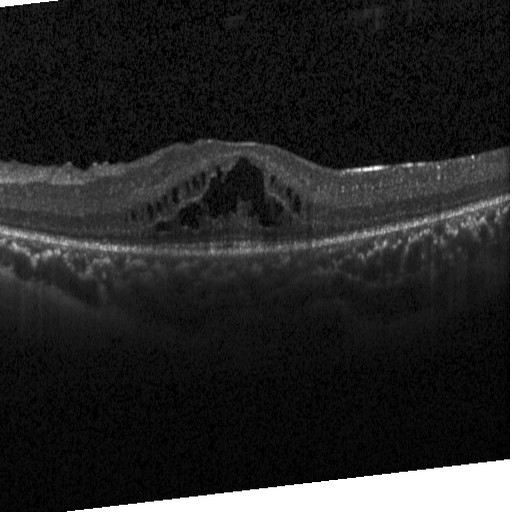
Macular OCT: diabetic macular edema (DME).